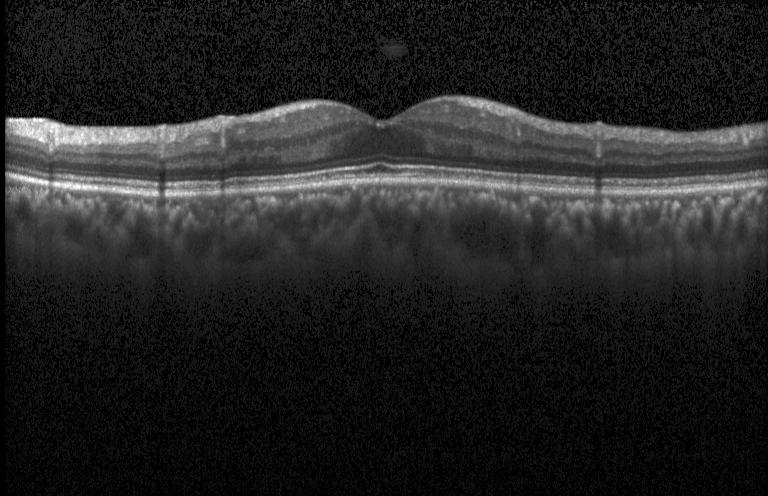 Macular OCT: neither choroidal neovascularization, diabetic macular edema, nor drusen.